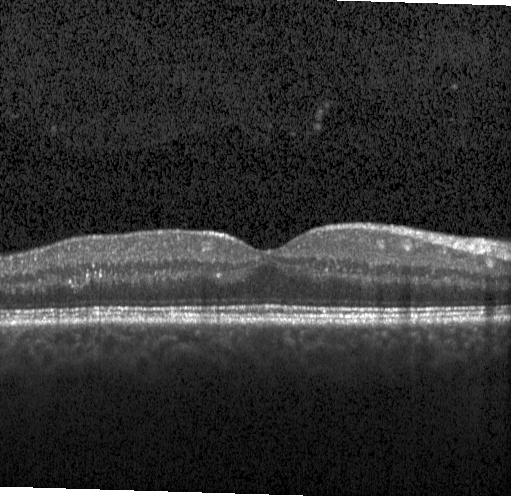

Finding: no evidence of CNV, DME, or drusen.